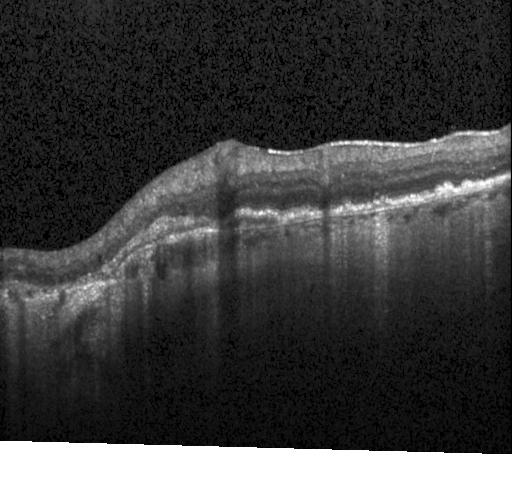

OCT B-scan; macular scan; spectral-domain OCT — The scan shows a choroidal neovascular membrane.